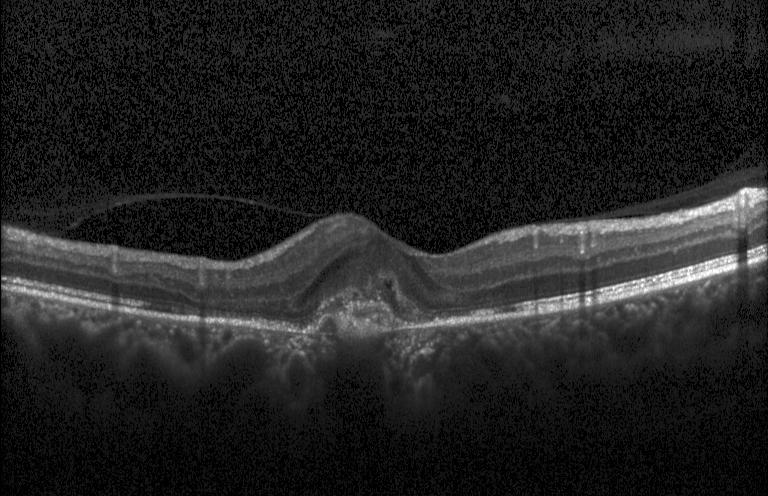
OCT B-scan; horizontal scan through the fovea; spectral-domain OCT — Macular OCT: choroidal neovascularization (CNV).